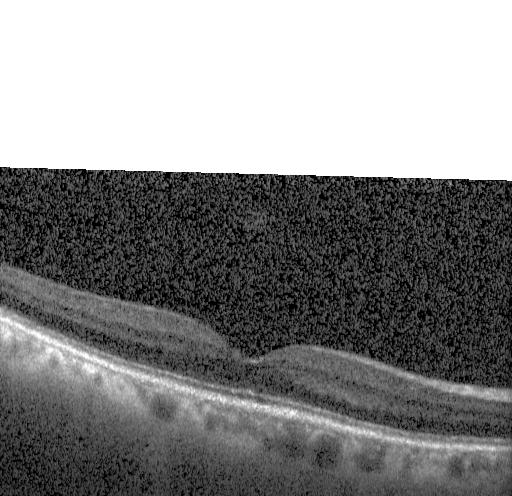

Optical coherence tomography scan
Macular OCT: no choroidal neovascularization, diabetic macular edema, or drusen.